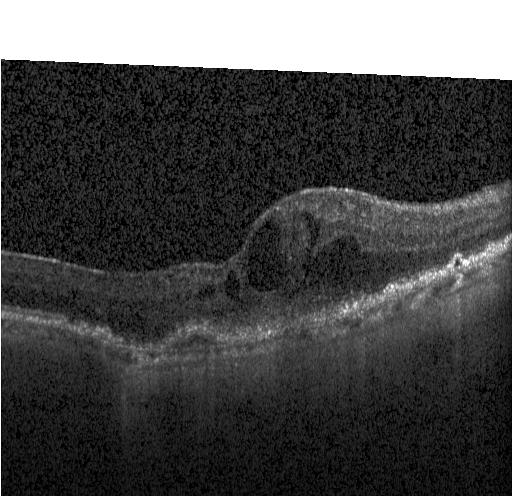

Retinal OCT cross-section — This B-scan demonstrates a choroidal neovascular membrane.